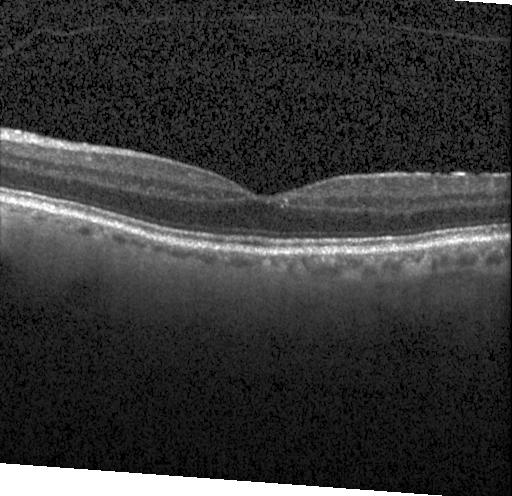
Heidelberg Spectralis OCT system, retinal OCT cross-section
Diagnosis: no choroidal neovascularization, diabetic macular edema, or drusen.